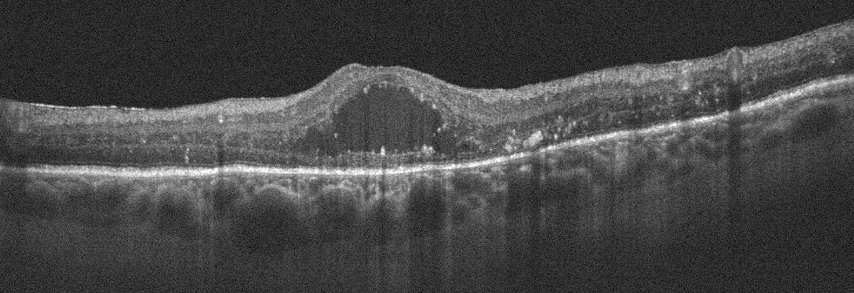
Optical coherence tomography B-scan. Right eye
This B-scan demonstrates DME.